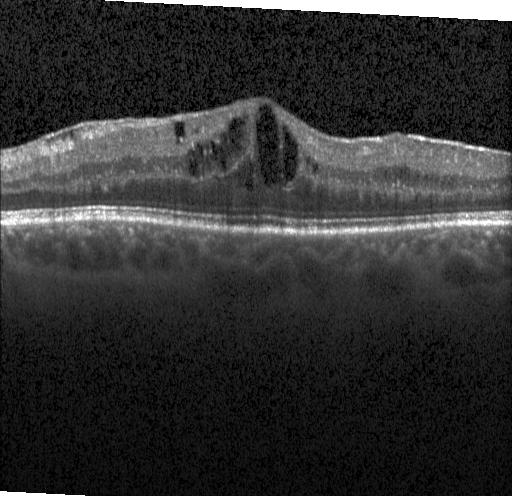 Retinal OCT B-scan. Acquired on a Heidelberg Spectralis — Macular OCT: diabetic macular edema (DME).